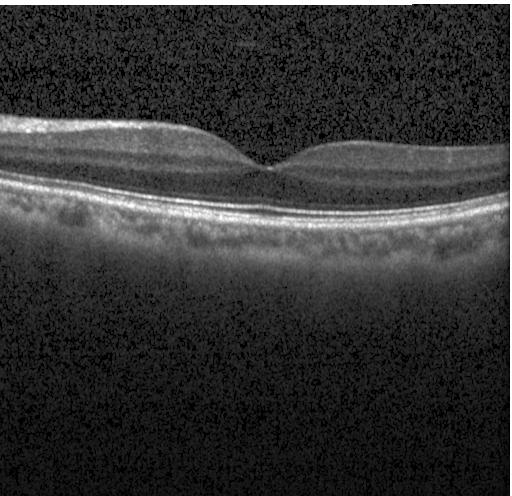

Retinal OCT B-scan, through the macula, acquired on a Heidelberg Spectralis, spectral-domain OCT.
No evidence of CNV, DME, or drusen.